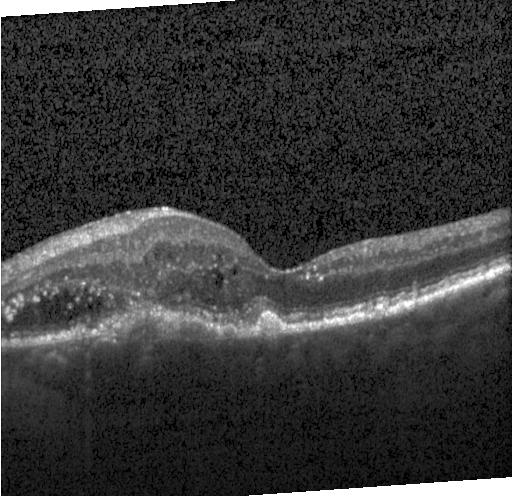 OCT line scan; horizontal scan through the fovea; Heidelberg Spectralis OCT system; SD-OCT. Choroidal neovascularization.